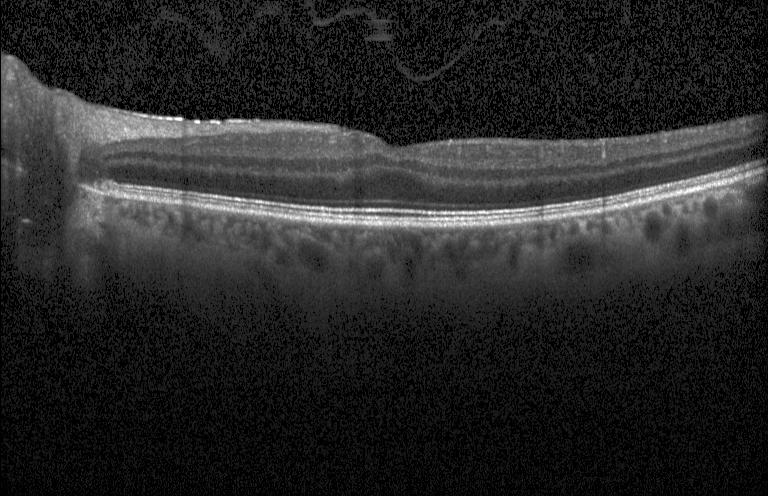
Macular scan · optical coherence tomography B-scan · spectral-domain OCT — OCT finding: no choroidal neovascularization, diabetic macular edema, or drusen.